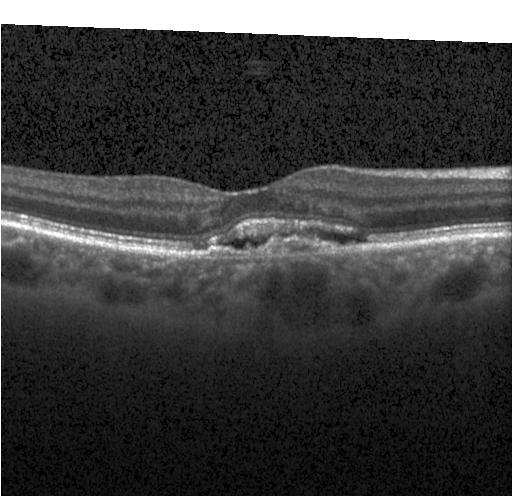
Choroidal neovascularization (CNV).